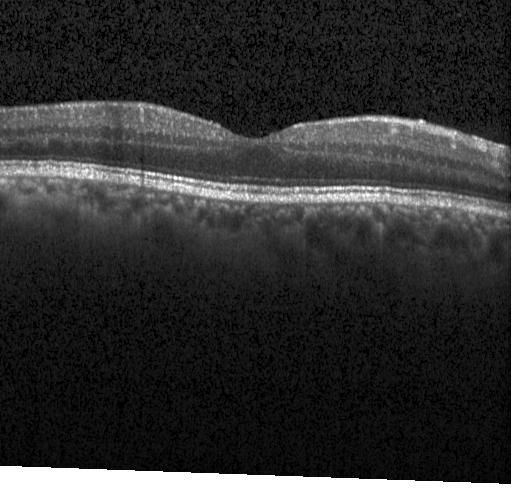

Optical coherence tomography scan · instrument: Heidelberg Spectralis · SD-OCT
Impression: no CNV, no DME, and no drusen.